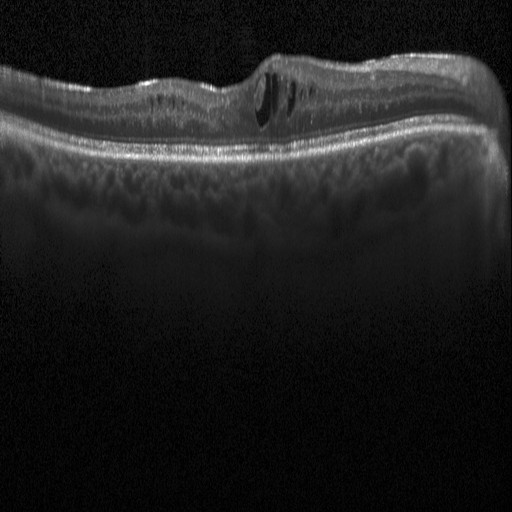 Finding: DME.